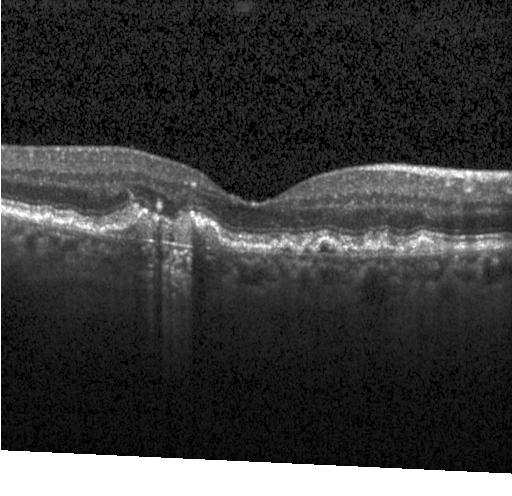 Macular scan, SD-OCT, retinal OCT cross-section, instrument: Heidelberg Spectralis — Finding: a choroidal neovascular membrane.